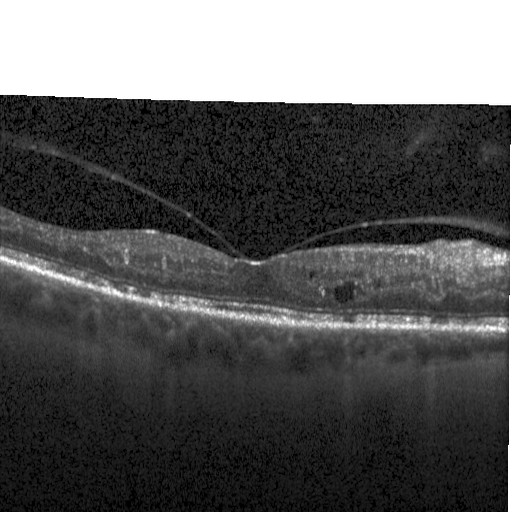

Retinal OCT cross-section · spectral-domain OCT. Finding: diabetic macular edema (DME).